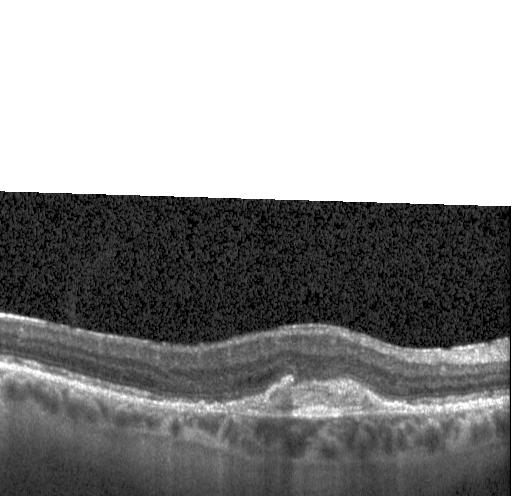

Finding: a choroidal neovascular membrane.